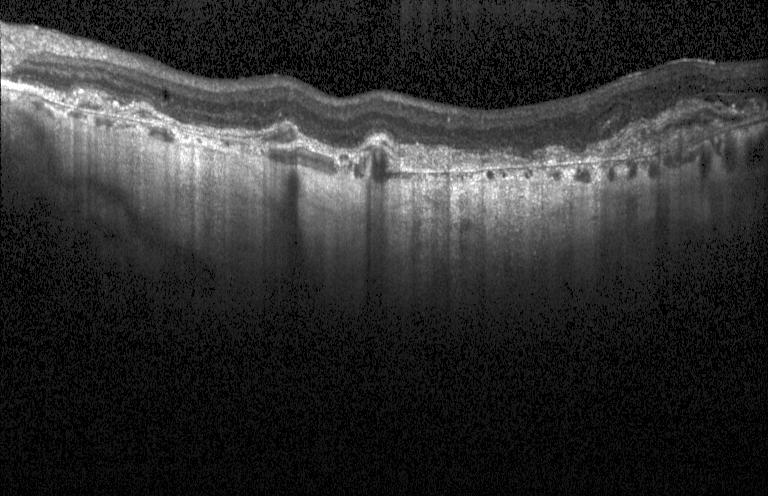 Spectral-domain OCT. Acquired on a Heidelberg Spectralis. OCT B-scan
Diagnosis: a choroidal neovascular membrane.